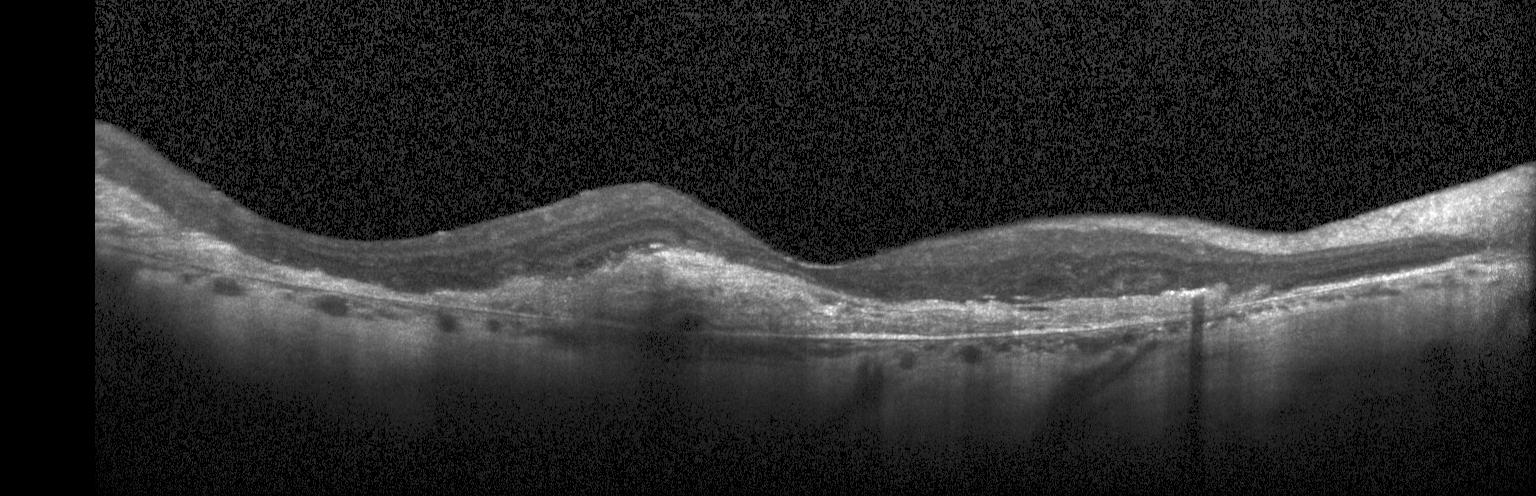

Spectral-domain optical coherence tomography · OCT B-scan · Heidelberg Spectralis · through the macula — Macular OCT: a choroidal neovascular membrane.